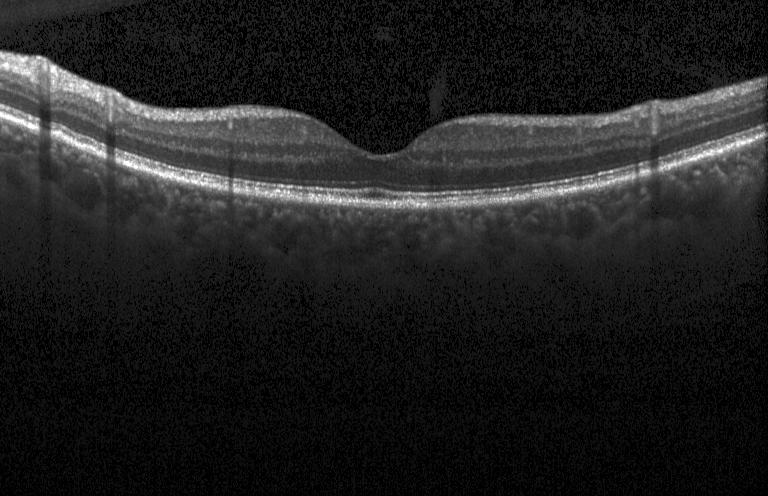 Diagnosis: no evidence of choroidal neovascularization, diabetic macular edema, or drusen.